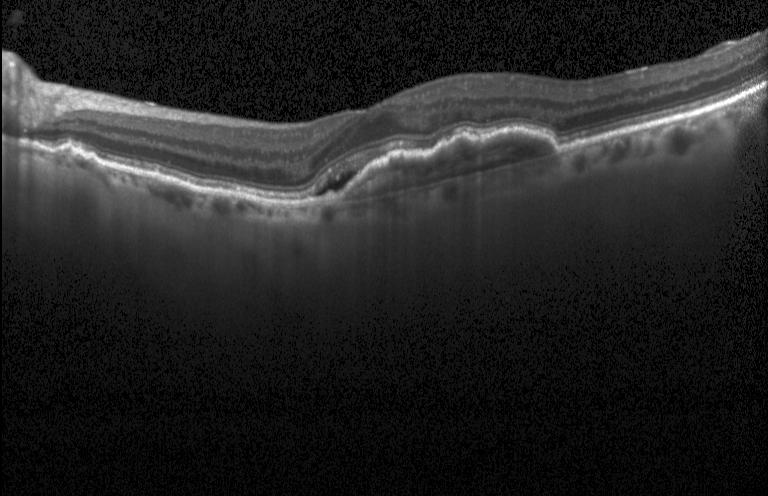

Finding: CNV.